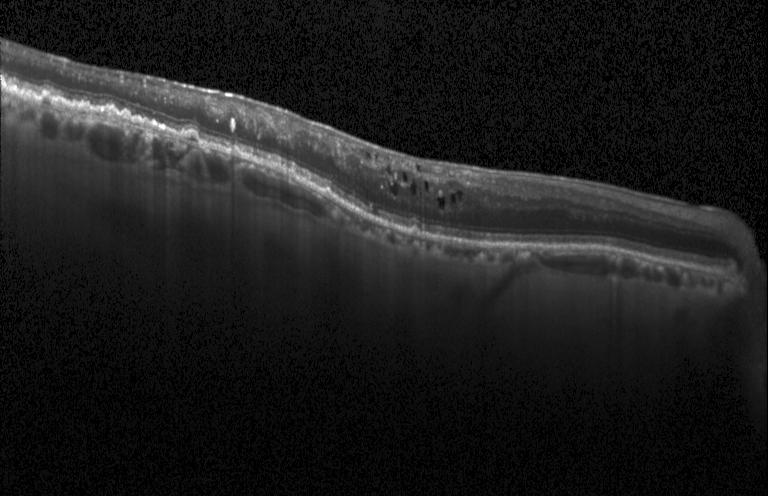 Optical coherence tomography B-scan · instrument: Heidelberg Spectralis · through the macula · SD-OCT
A choroidal neovascular membrane.